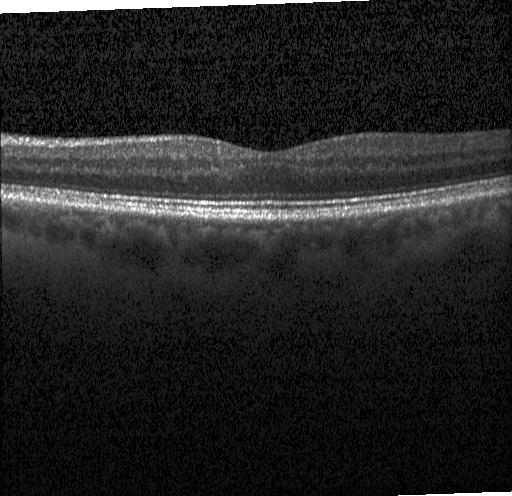
OCT line scan — Diagnosis: no choroidal neovascularization, no diabetic macular edema, and no drusen.